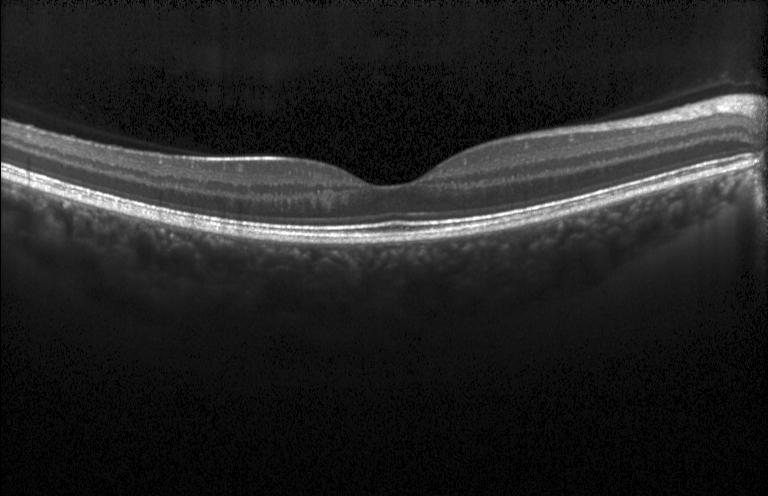 Acquired on a Heidelberg Spectralis · OCT line scan · SD-OCT.
Finding: neither CNV, DME, nor drusen.